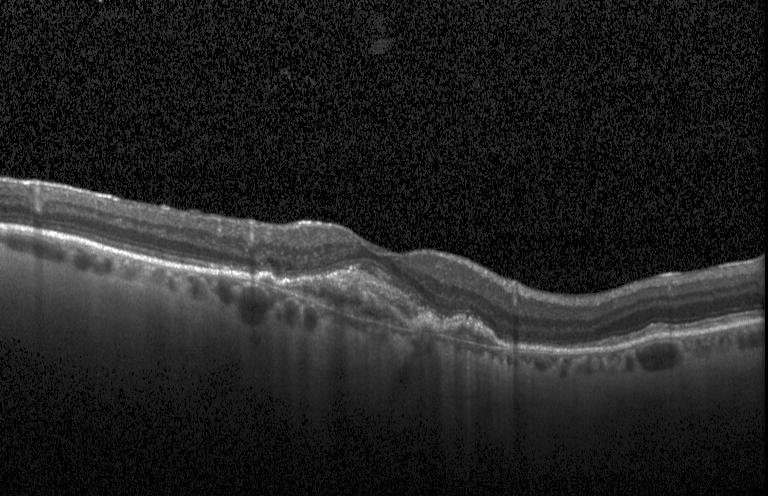
Optical coherence tomography scan, fovea-centered
OCT finding: a choroidal neovascular membrane.